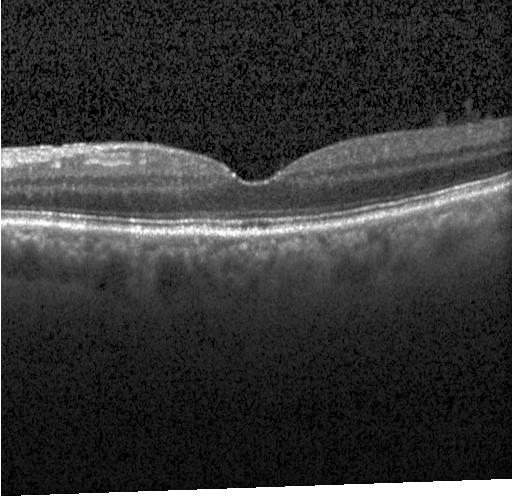
OCT B-scan · Heidelberg Spectralis · spectral-domain optical coherence tomography · macular scan
Macular OCT: neither choroidal neovascularization, diabetic macular edema, nor drusen.